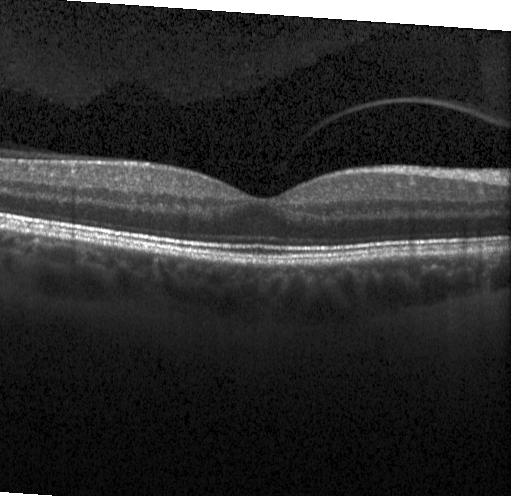 Macular OCT: no CNV, no DME, and no drusen.